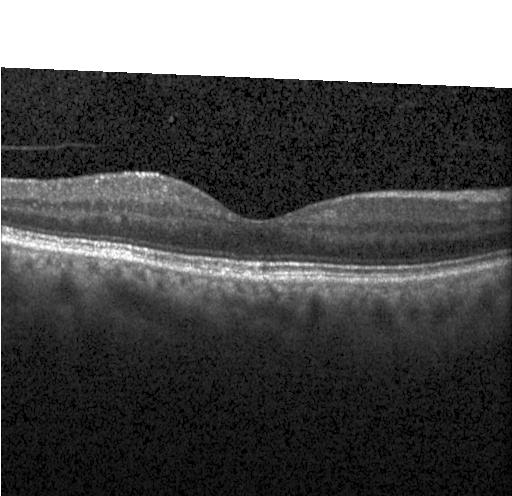

Optical coherence tomography scan.
Macular OCT: neither choroidal neovascularization, diabetic macular edema, nor drusen.